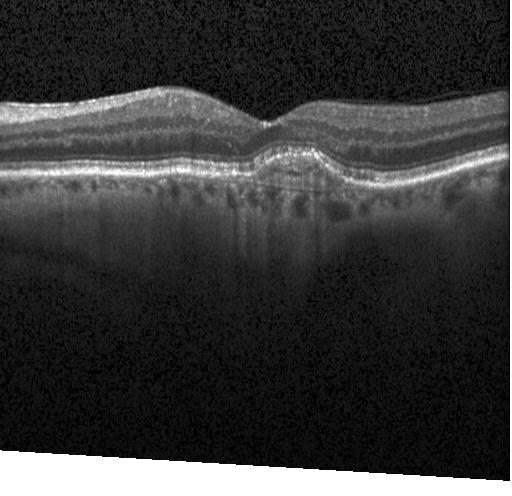
SD-OCT; optical coherence tomography B-scan; acquired on a Heidelberg Spectralis
Assessment: a choroidal neovascular membrane.